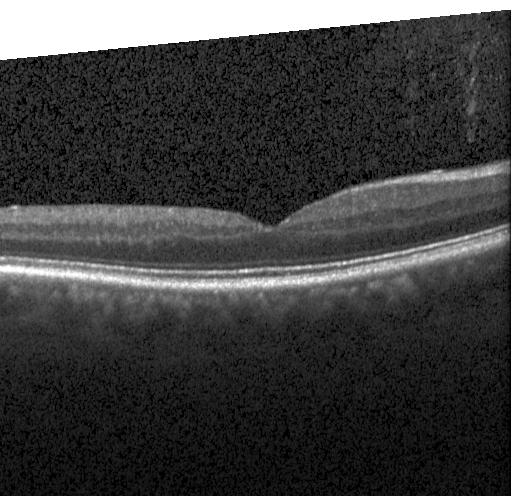 OCT line scan, macular scan, Heidelberg Spectralis OCT system, spectral-domain optical coherence tomography
Impression: no CNV, no DME, and no drusen.